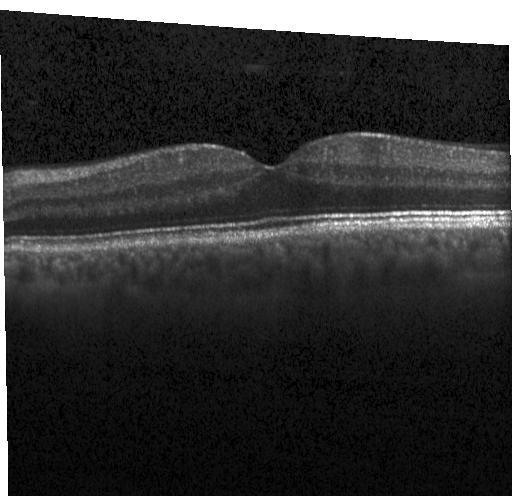
Heidelberg Spectralis OCT system · SD-OCT · optical coherence tomography B-scan — This B-scan demonstrates neither choroidal neovascularization, diabetic macular edema, nor drusen.